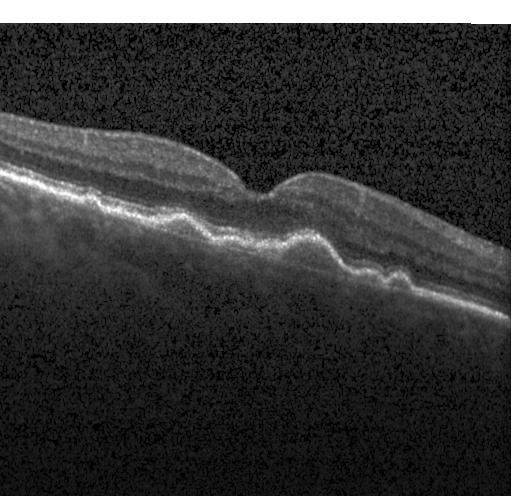
OCT scan showing choroidal neovascularization.